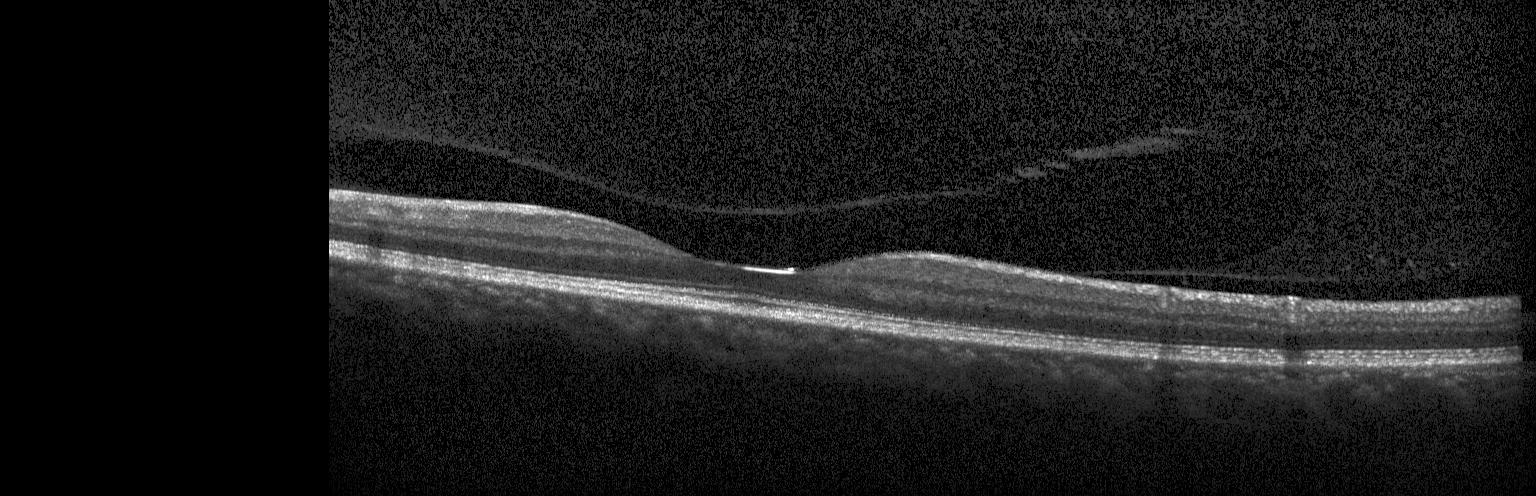 Optical coherence tomography B-scan, centered on the fovea, Heidelberg Spectralis — The scan shows neither choroidal neovascularization, diabetic macular edema, nor drusen.